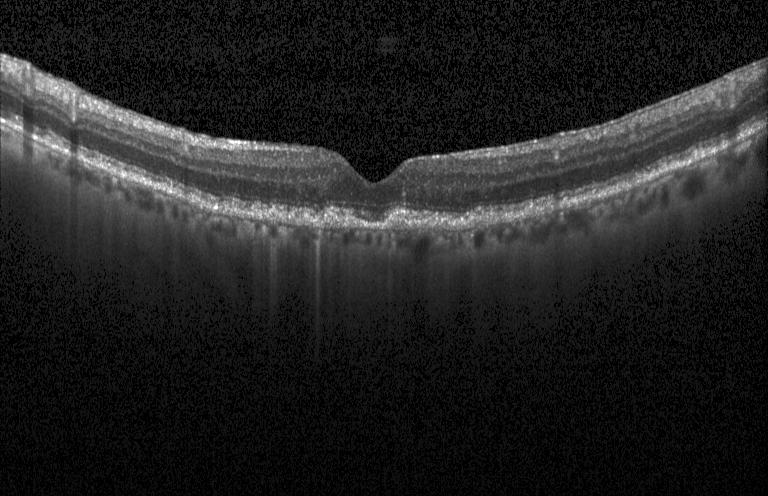

Impression: drusen.